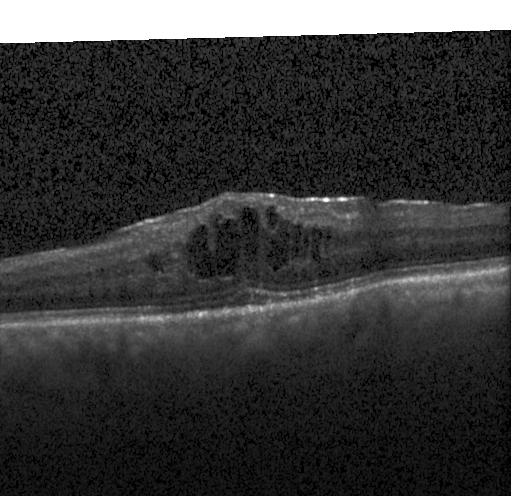

Optical coherence tomography B-scan — Finding: diabetic macular edema.